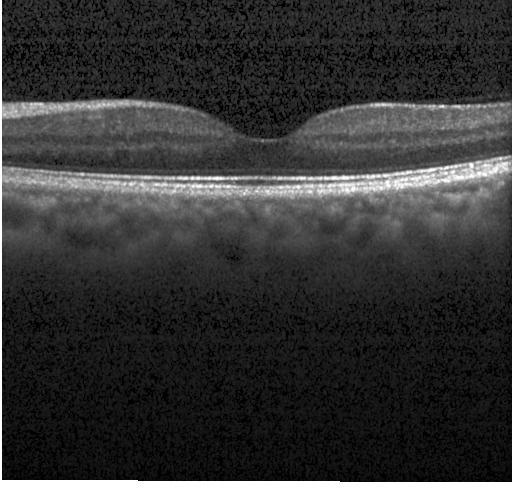
OCT finding: neither choroidal neovascularization, diabetic macular edema, nor drusen.